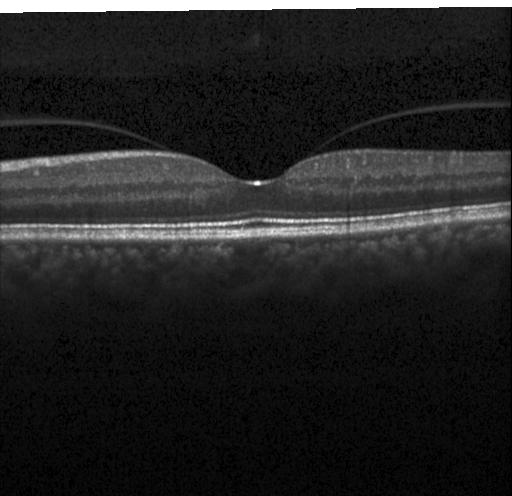

Fovea-centered. Heidelberg Spectralis OCT system. OCT B-scan — Finding: neither CNV, DME, nor drusen.